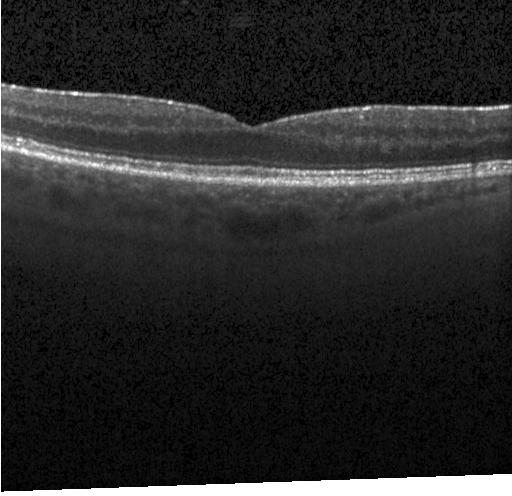

Optical coherence tomography scan.
Assessment: no evidence of choroidal neovascularization, diabetic macular edema, or drusen.